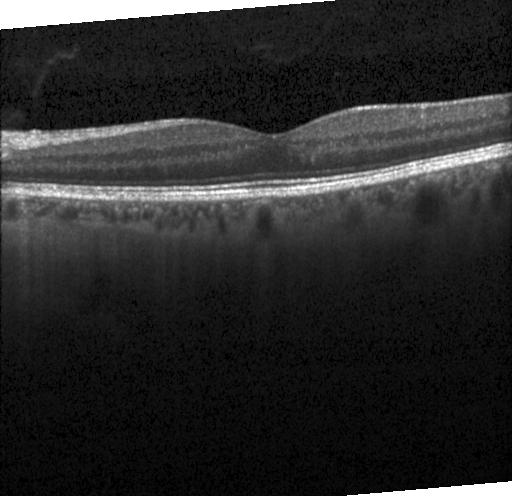
OCT B-scan; Heidelberg Spectralis; fovea-centered; SD-OCT. Diagnosis: no evidence of choroidal neovascularization, diabetic macular edema, or drusen.